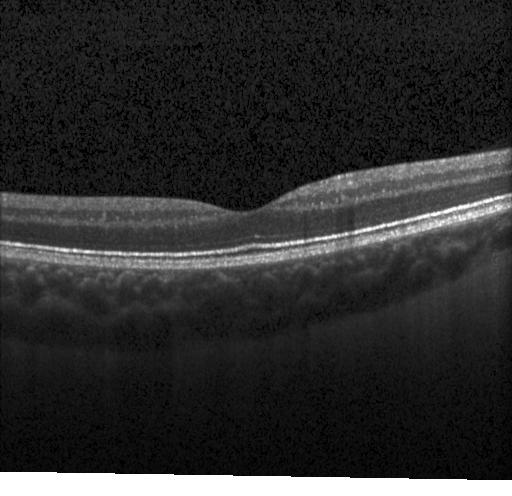
Retinal OCT B-scan.
Diagnosis: no choroidal neovascularization, diabetic macular edema, or drusen.